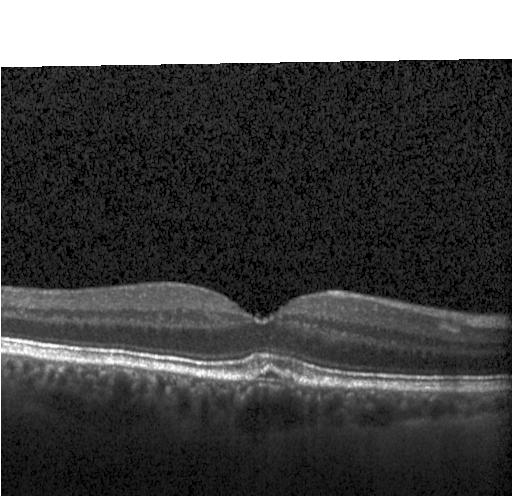

Spectral-domain OCT B-scan: CNV.